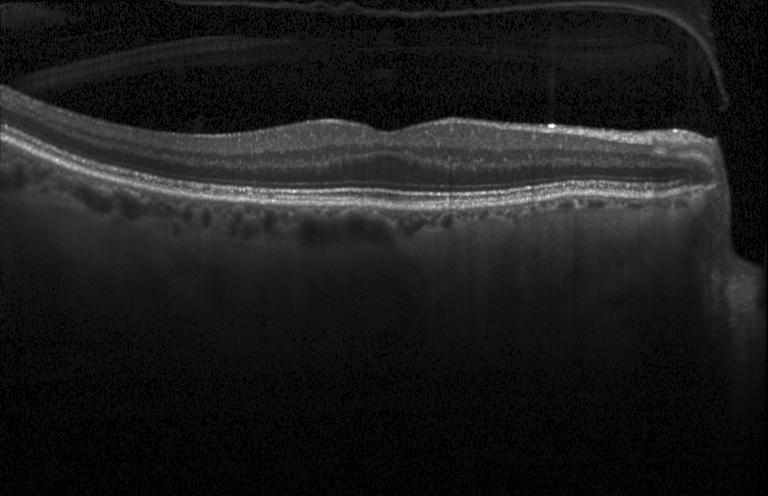

Optical coherence tomography B-scan. SD-OCT. This B-scan demonstrates no CNV, DME, or drusen.